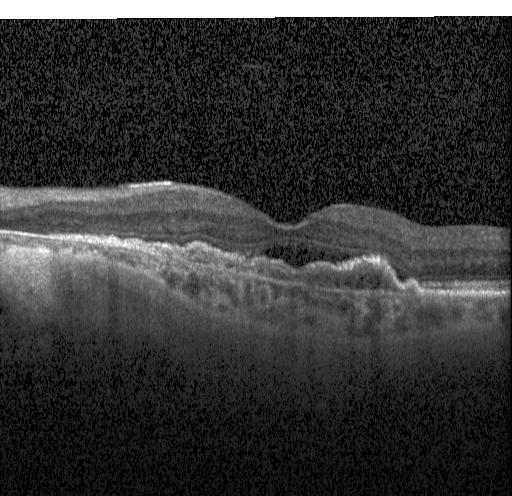 Macular OCT demonstrating choroidal neovascularization (CNV).